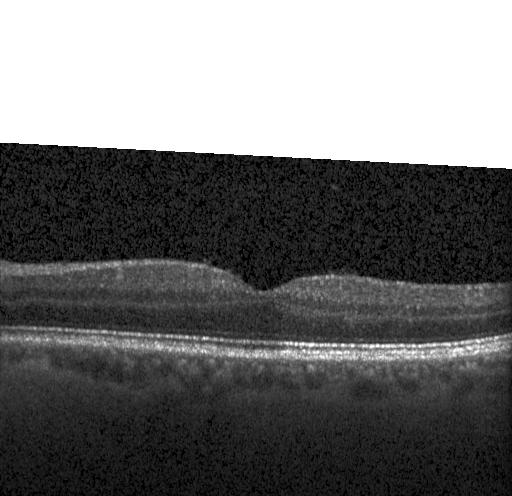
OCT B-scan showing no evidence of choroidal neovascularization, diabetic macular edema, or drusen.